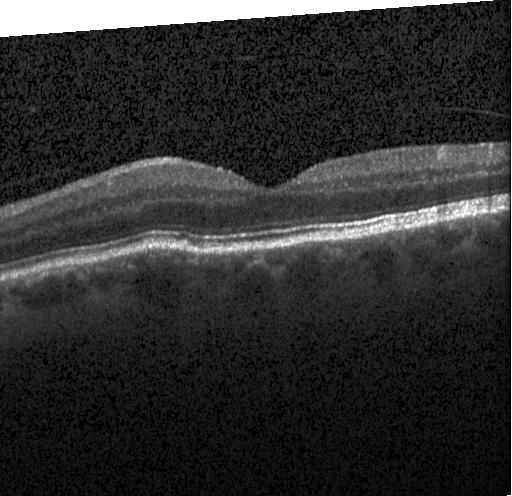

SD-OCT · retinal OCT B-scan — Dx: neither choroidal neovascularization, diabetic macular edema, nor drusen.